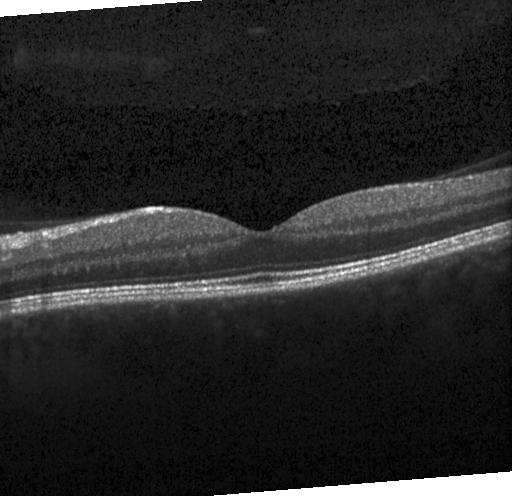
Spectral-domain optical coherence tomography · retinal OCT cross-section · acquired on a Heidelberg Spectralis — No CNV, DME, or drusen.